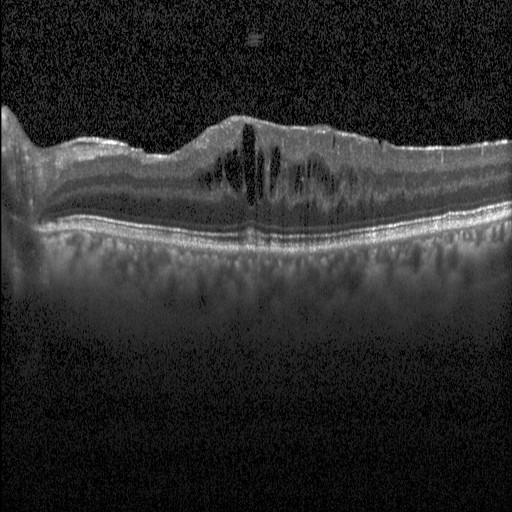

OCT finding: diabetic macular edema (DME).